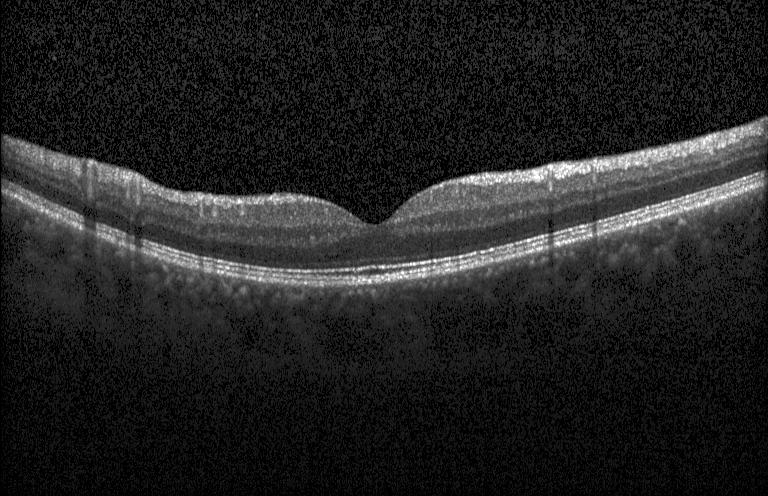
Spectral-domain OCT, retinal OCT B-scan, macular scan
No choroidal neovascularization, diabetic macular edema, or drusen.